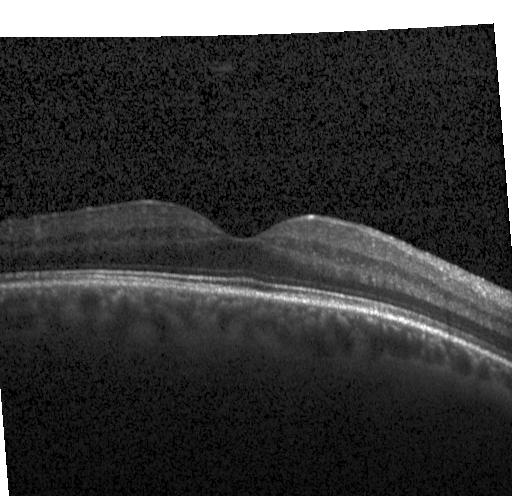 Spectral-domain OCT B-scan: no choroidal neovascularization, diabetic macular edema, or drusen.